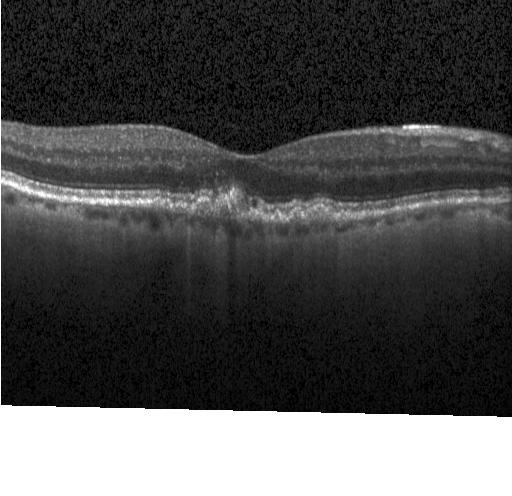
Retinal OCT B-scan.
Multiple drusen.